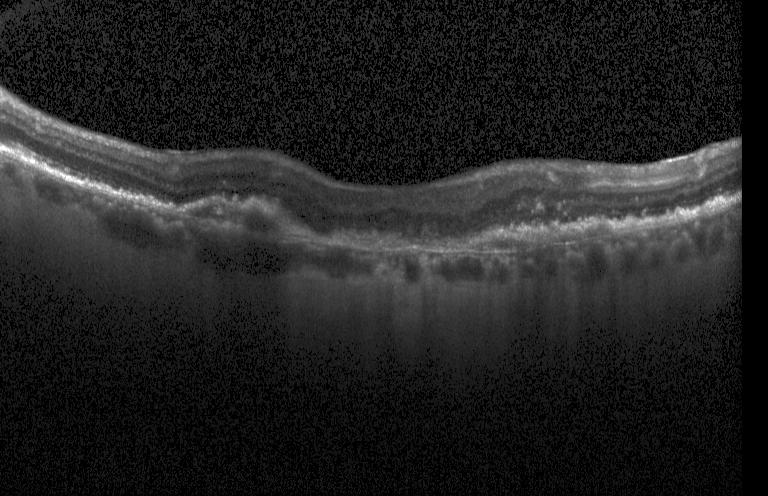

Dx: choroidal neovascularization (CNV).